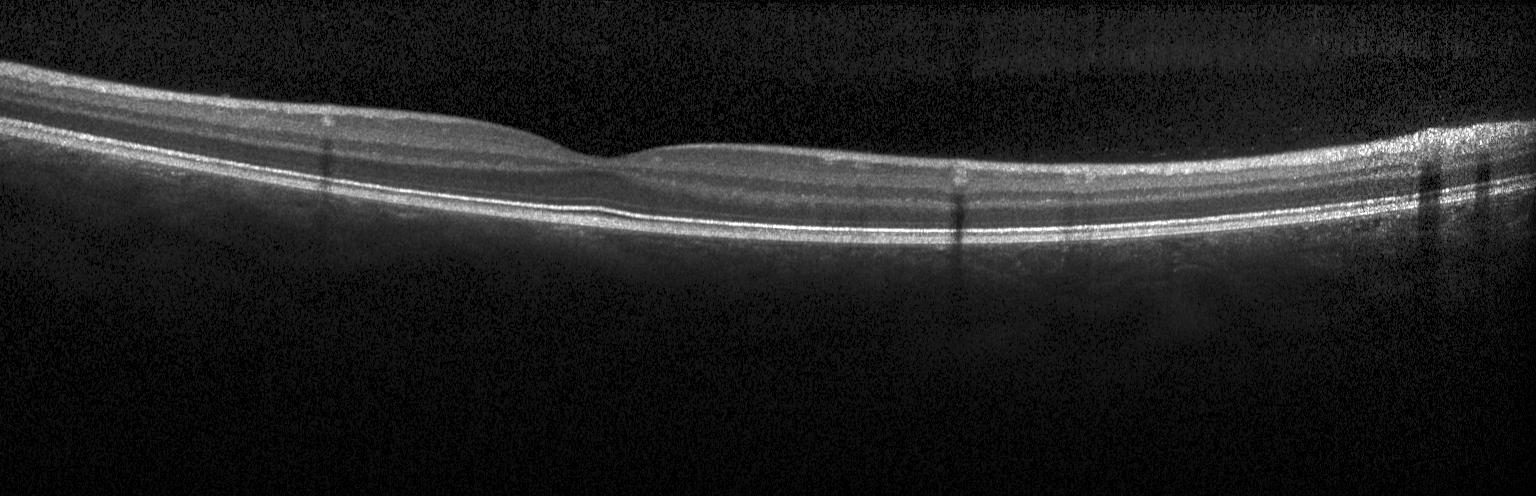
Macular scan; OCT line scan; Heidelberg Spectralis; SD-OCT. This B-scan demonstrates neither CNV, DME, nor drusen.